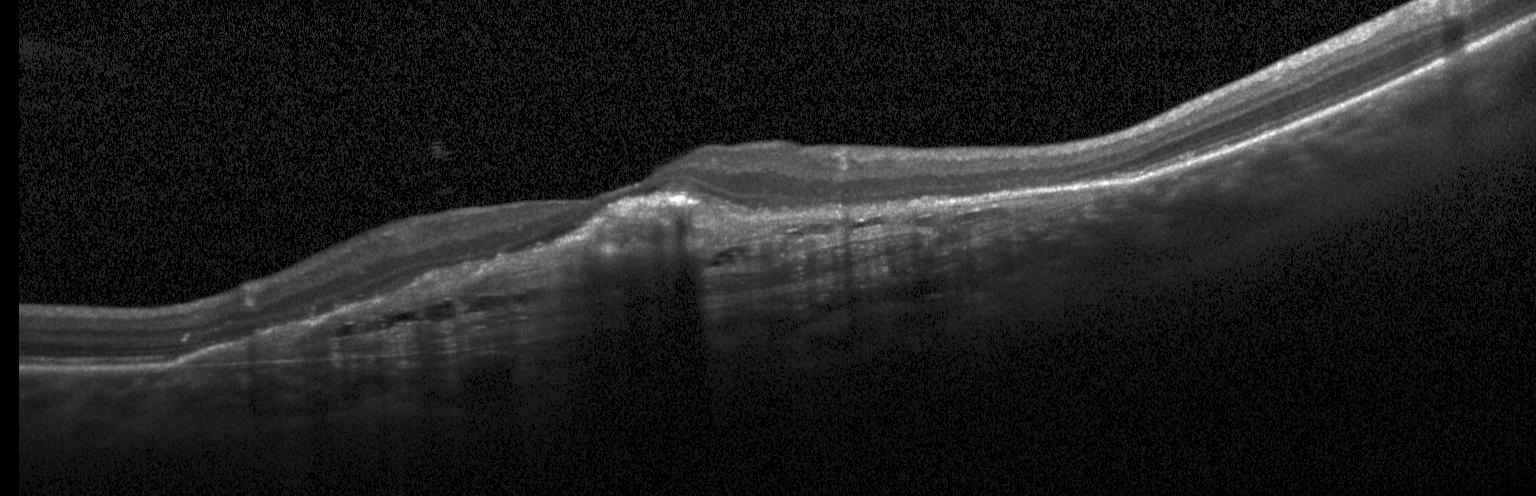
Spectral-domain OCT B-scan: a choroidal neovascular membrane.